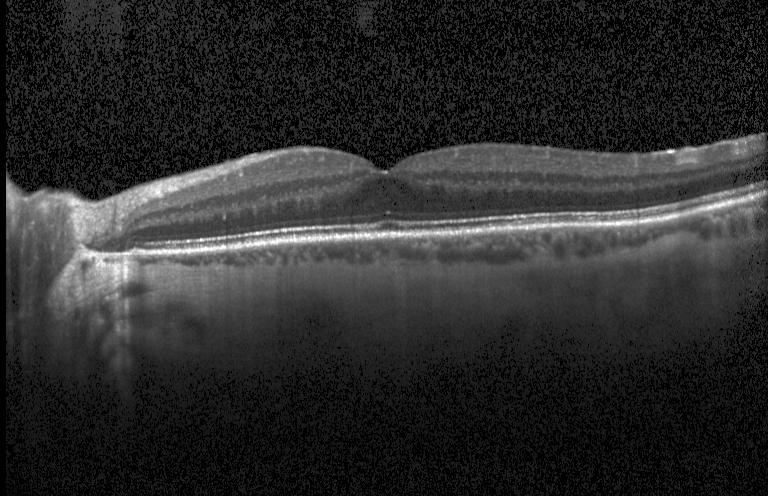 Impression: no CNV, DME, or drusen.